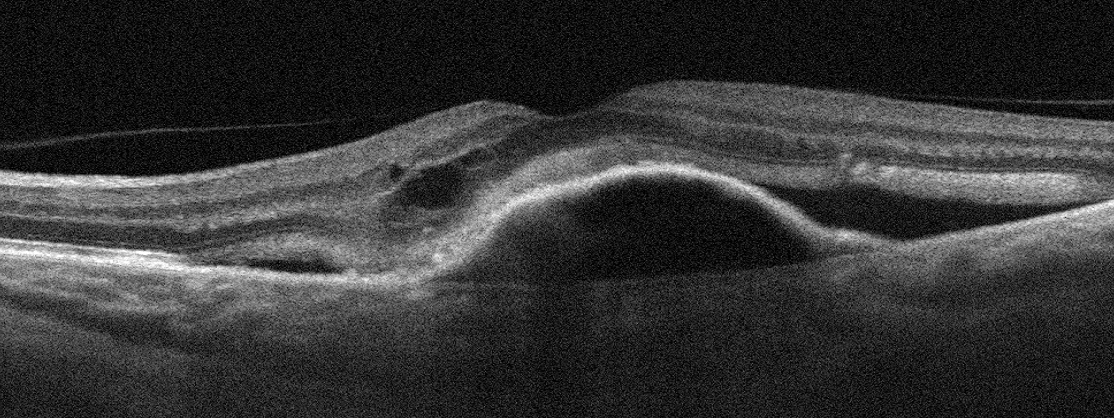
Dx: AMD.